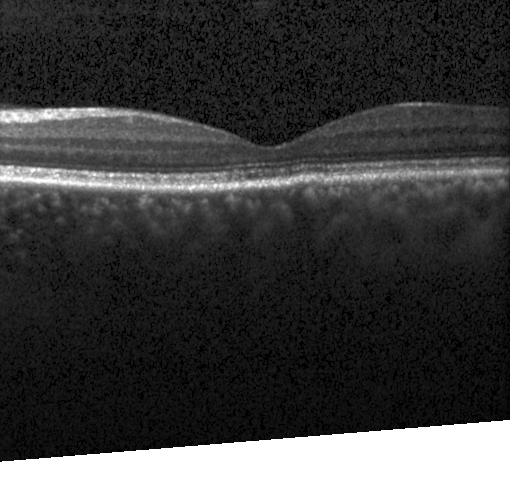

Retinal OCT cross-section; macular scan
The scan shows neither choroidal neovascularization, diabetic macular edema, nor drusen.